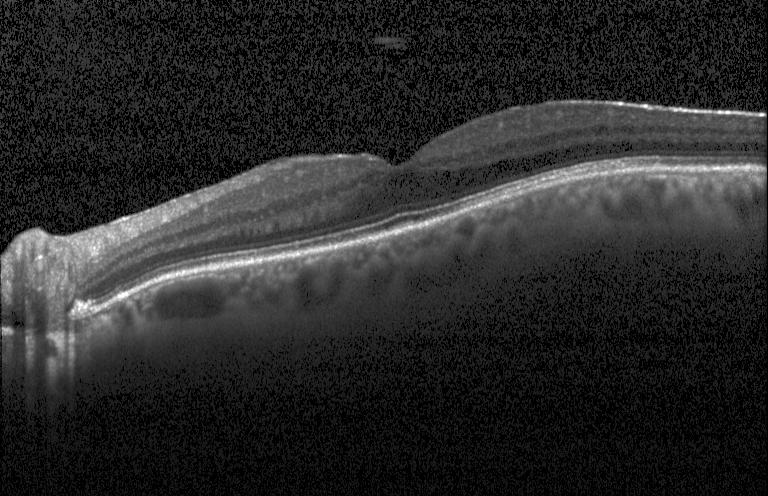
Fovea-centered · retinal OCT B-scan — Finding: no choroidal neovascularization, no diabetic macular edema, and no drusen.